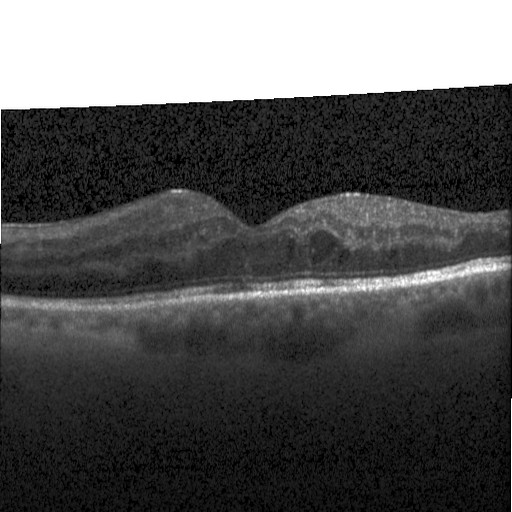 Impression: DME.